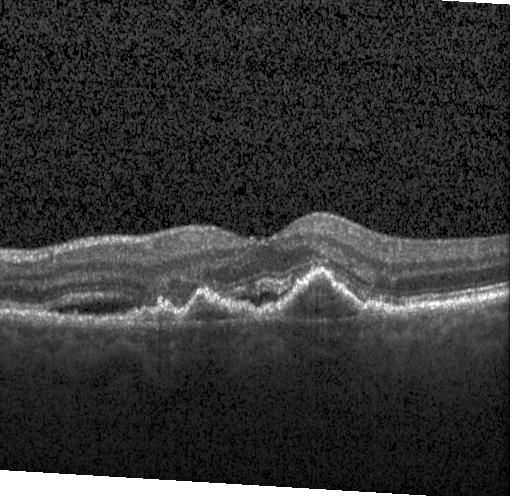 Diagnosis: a choroidal neovascular membrane.